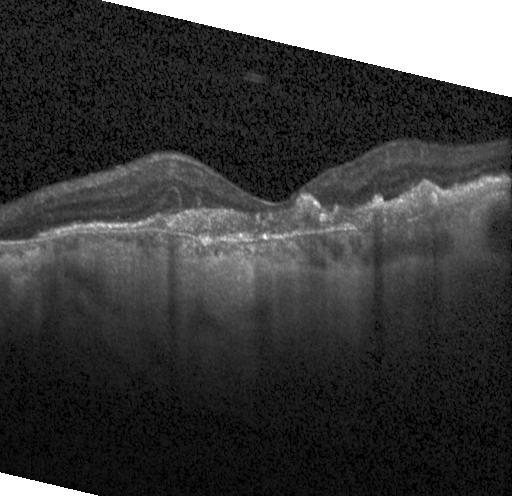

OCT line scan
Impression: a choroidal neovascular membrane.